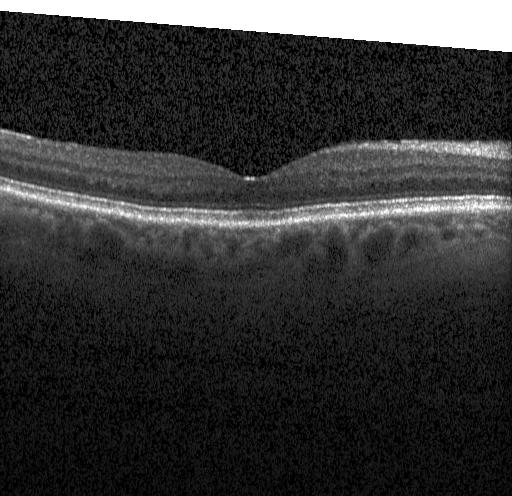 This B-scan demonstrates no evidence of choroidal neovascularization, diabetic macular edema, or drusen.